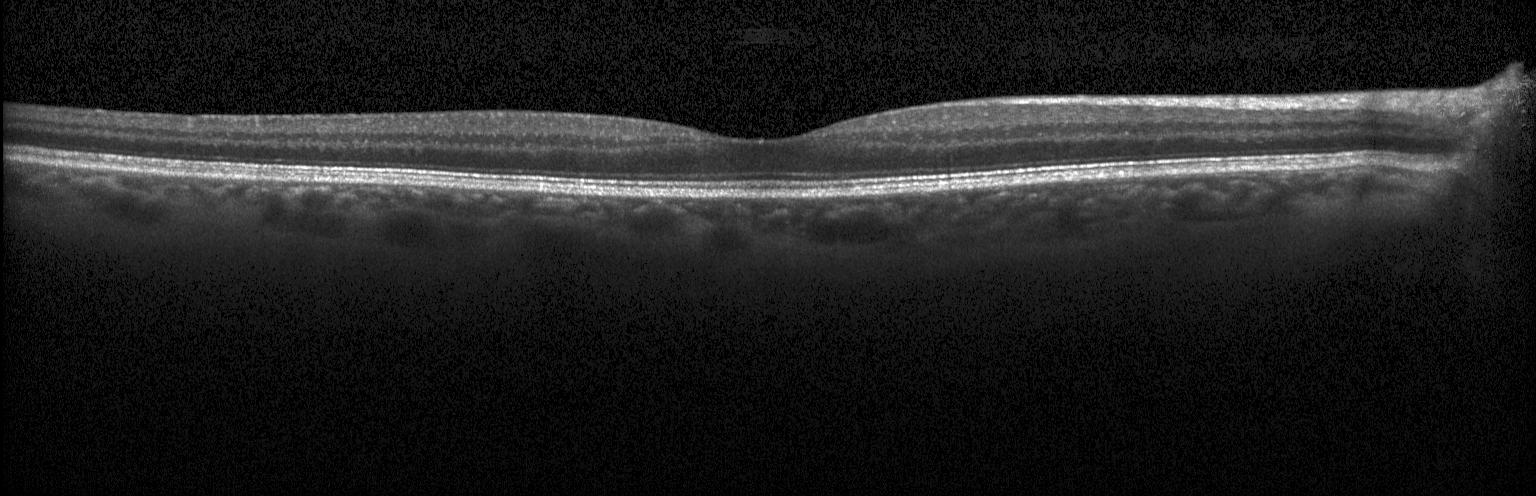

Retinal OCT B-scan. Instrument: Heidelberg Spectralis. Dx: neither CNV, DME, nor drusen.